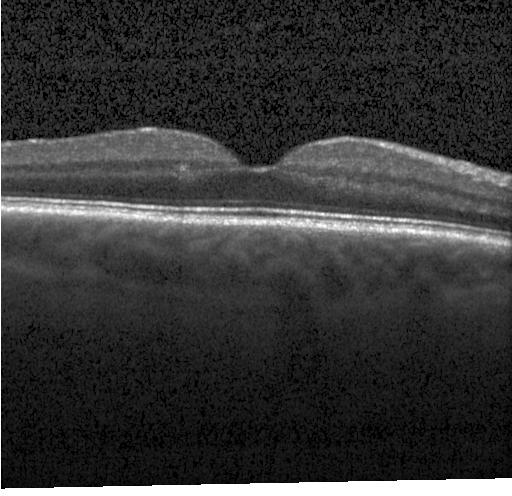 OCT line scan, acquired on a Heidelberg Spectralis — Diagnosis: neither choroidal neovascularization, diabetic macular edema, nor drusen.